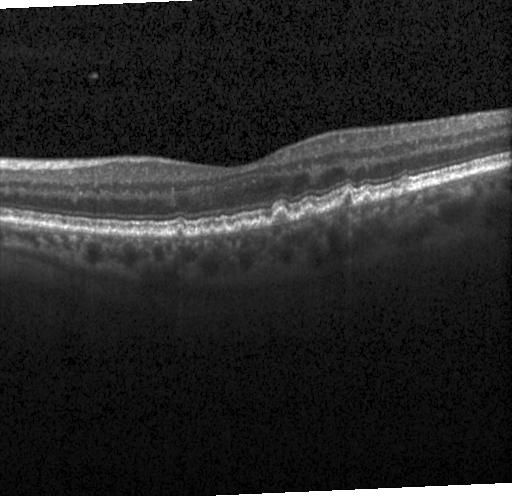 This B-scan demonstrates drusen.